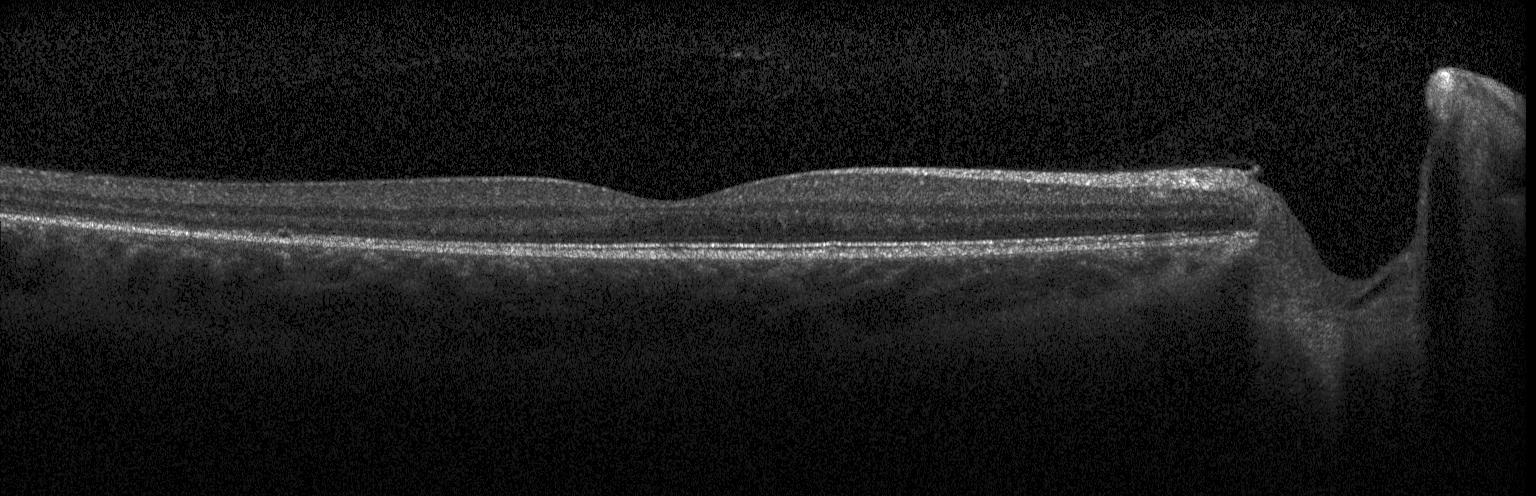 Optical coherence tomography scan; acquired on a Heidelberg Spectralis; spectral-domain optical coherence tomography
Impression: neither choroidal neovascularization, diabetic macular edema, nor drusen.